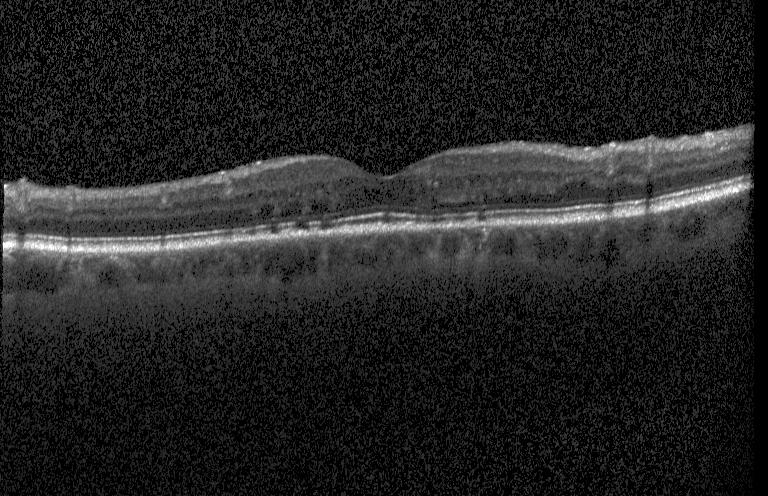

Optical coherence tomography B-scan; instrument: Heidelberg Spectralis
Macular OCT: DME.